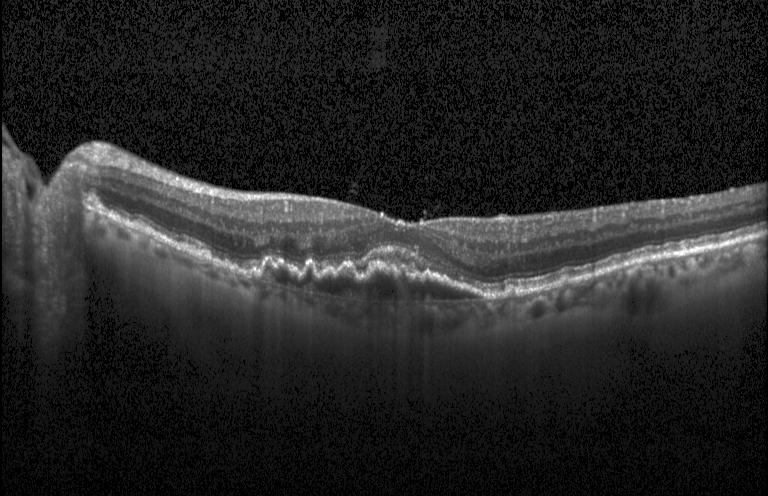 Retinal OCT cross-section showing a choroidal neovascular membrane.